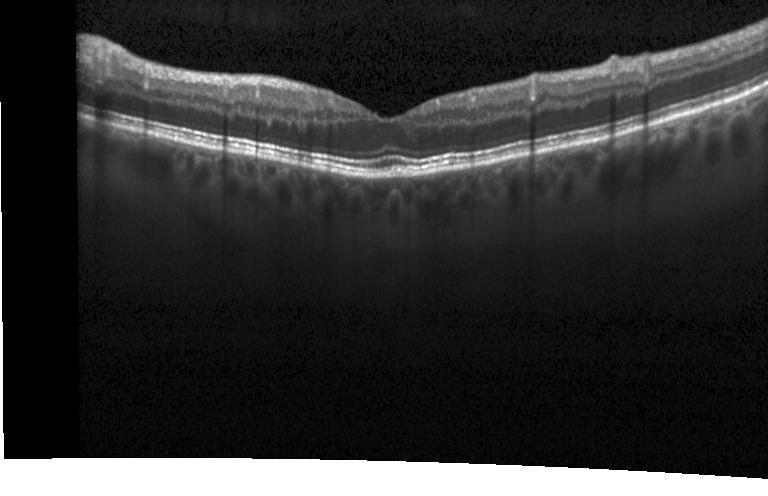 OCT B-scan showing no evidence of choroidal neovascularization, diabetic macular edema, or drusen.